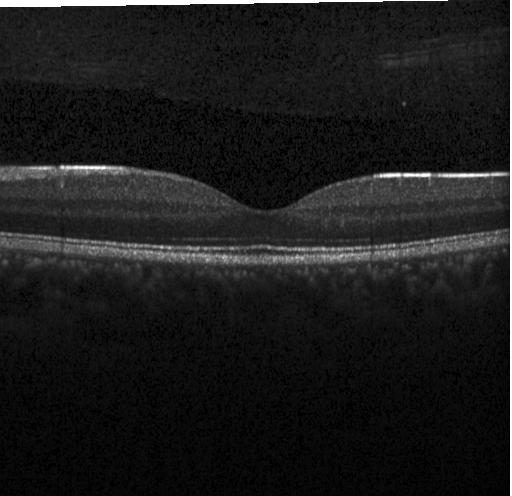
Retinal OCT cross-section; SD-OCT — Finding: no CNV, DME, or drusen.